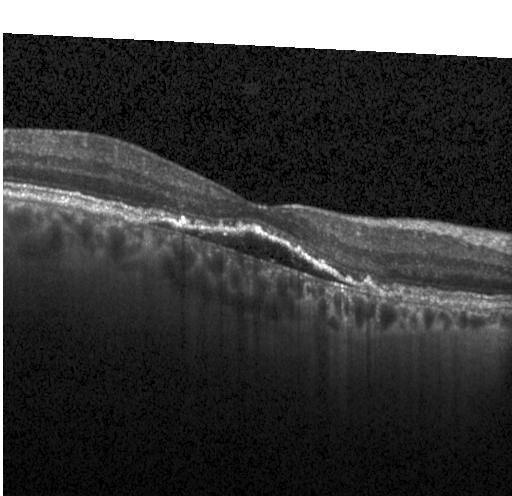

Impression: CNV.